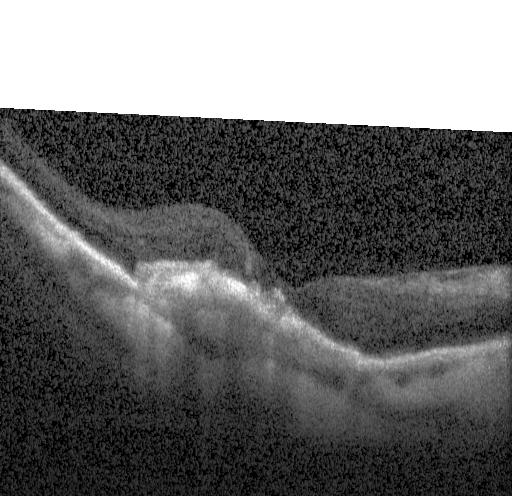 Diagnosis: a choroidal neovascular membrane.